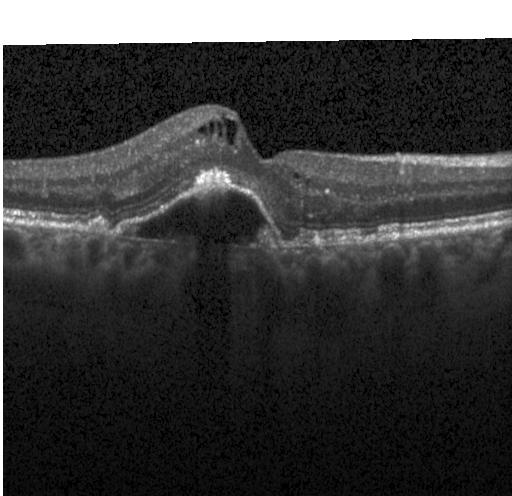

Retinal OCT B-scan.
Diagnosis: a choroidal neovascular membrane.